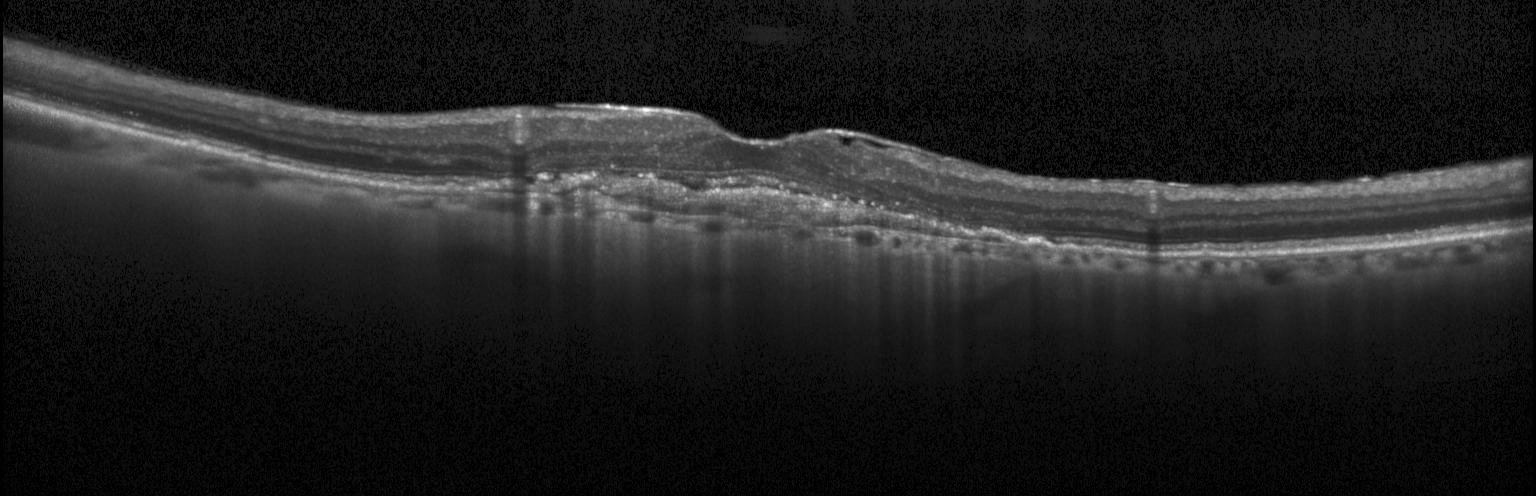

Dx: a choroidal neovascular membrane.